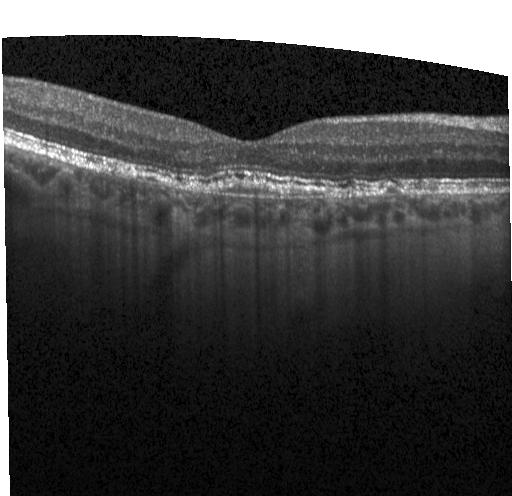

Retinal OCT B-scan, Heidelberg Spectralis OCT system. Dx: a choroidal neovascular membrane.